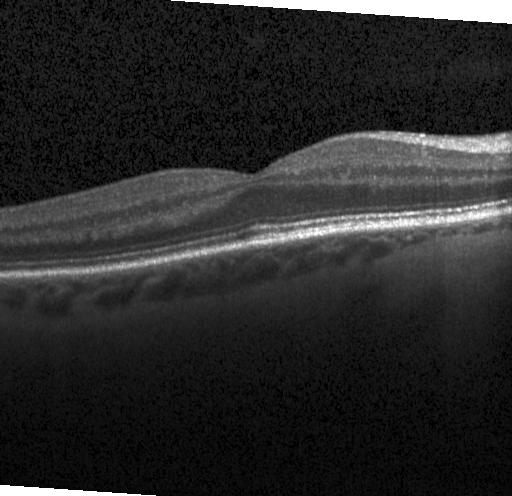 Optical coherence tomography scan.
Dx: no CNV, no DME, and no drusen.